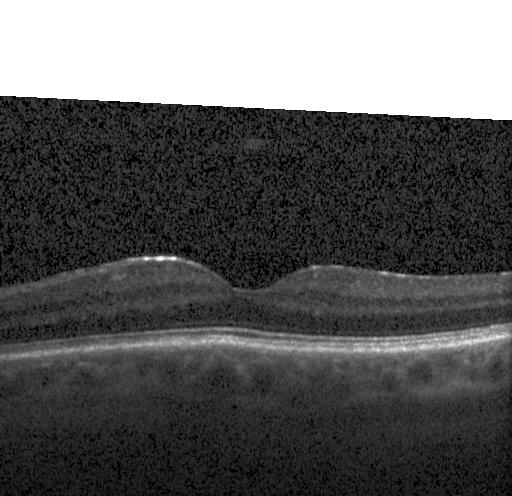
OCT B-scan showing neither CNV, DME, nor drusen.